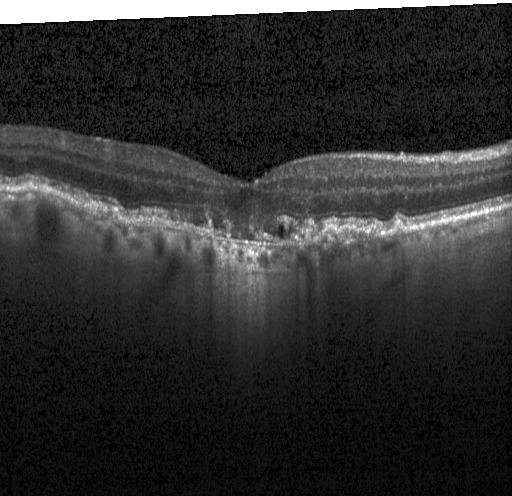

Macular scan, OCT line scan — Diagnosis: choroidal neovascularization.